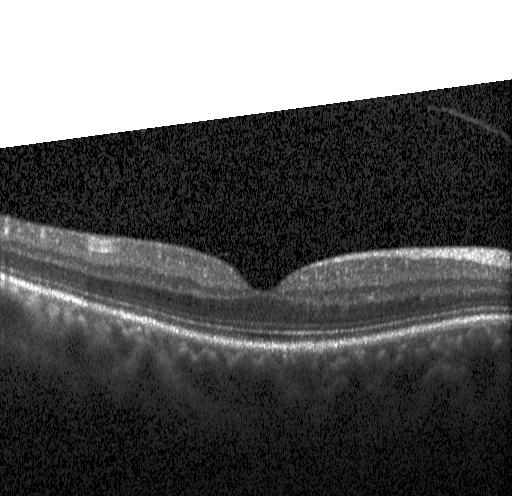
Retinal OCT cross-section. This B-scan demonstrates no choroidal neovascularization, diabetic macular edema, or drusen.